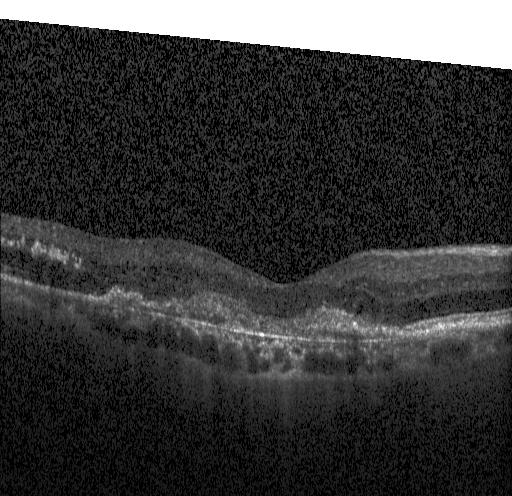

Macular OCT: choroidal neovascularization (CNV).